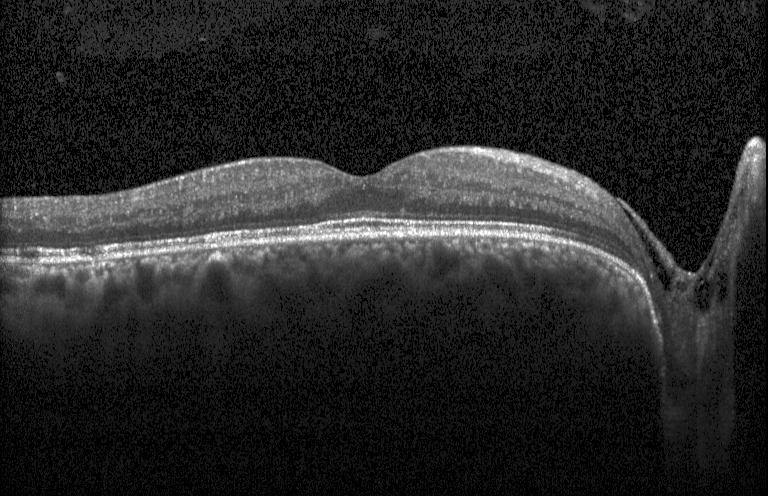 Impression: no choroidal neovascularization, diabetic macular edema, or drusen.